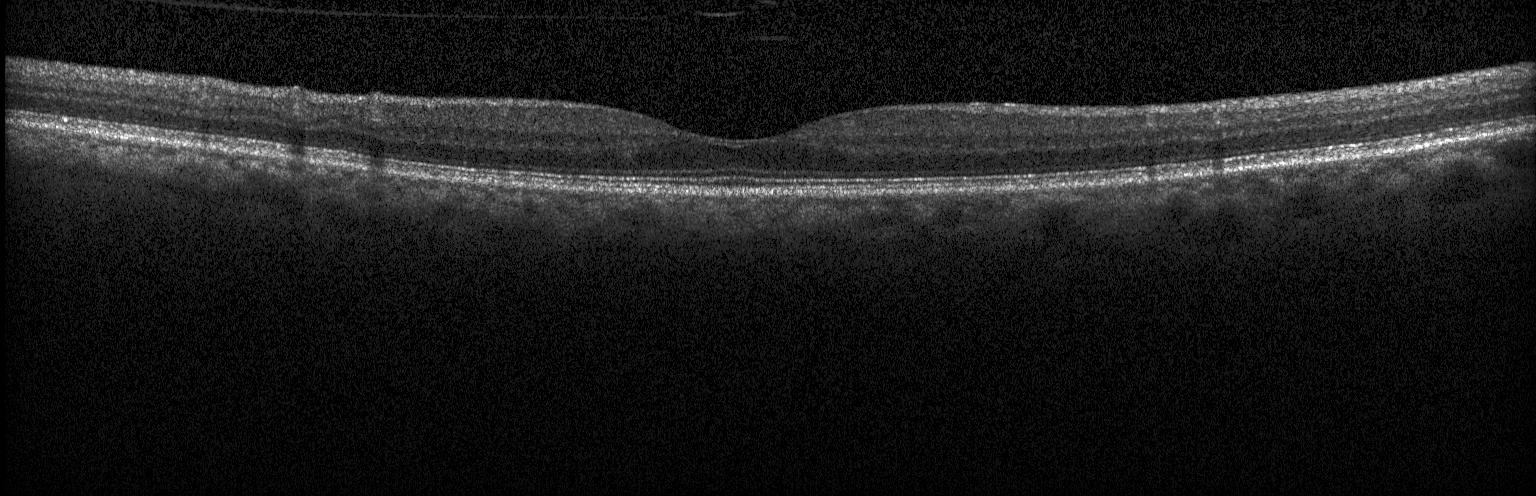

OCT line scan; Heidelberg Spectralis OCT system; fovea-centered; spectral-domain optical coherence tomography. Finding: no CNV, no DME, and no drusen.